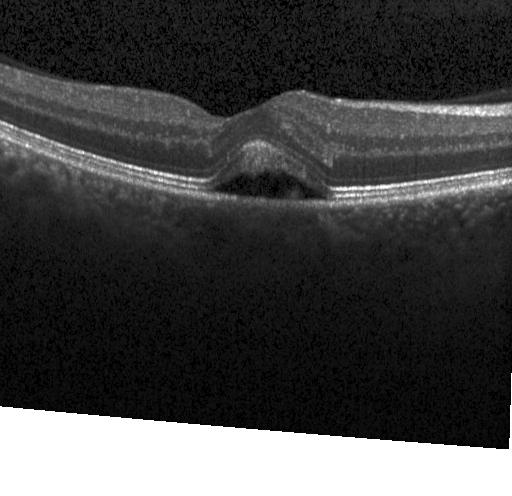

Heidelberg Spectralis OCT system · spectral-domain optical coherence tomography · OCT line scan
The scan shows CNV.